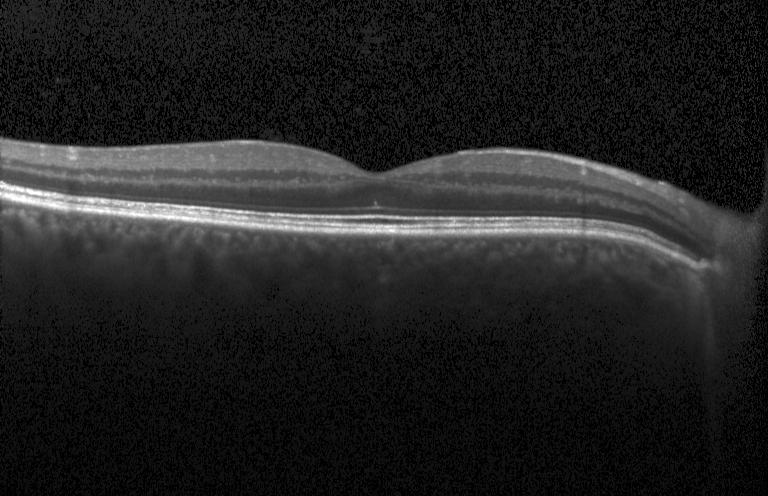
Spectral-domain OCT. Horizontal scan through the fovea. Optical coherence tomography scan.
Finding: neither choroidal neovascularization, diabetic macular edema, nor drusen.